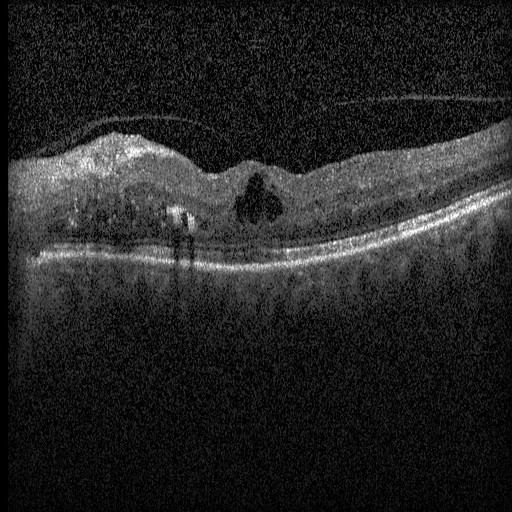 Fovea-centered. Optical coherence tomography scan — The scan shows diabetic macular edema (DME).